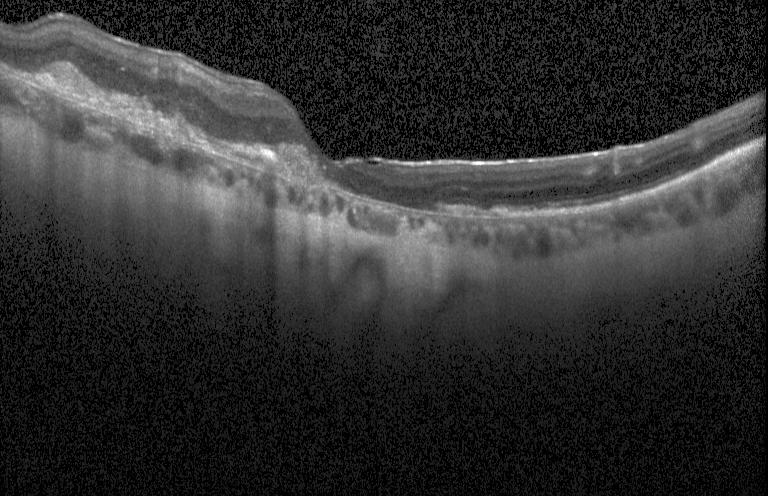 OCT B-scan. Impression: choroidal neovascularization.